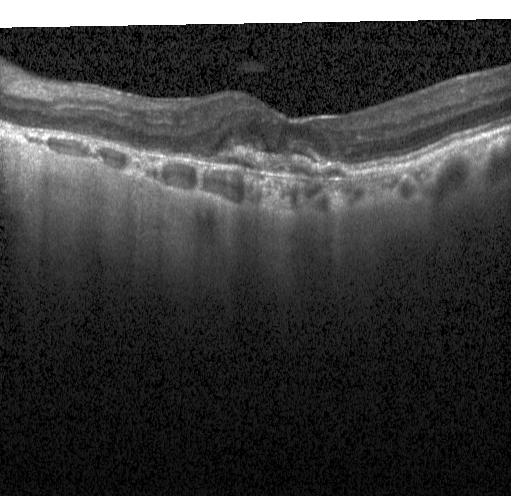 Finding: a choroidal neovascular membrane.